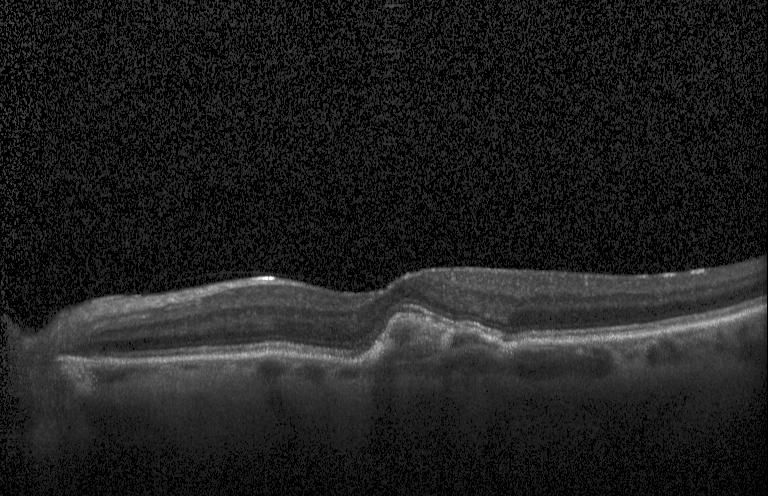

OCT scan showing choroidal neovascularization (CNV).